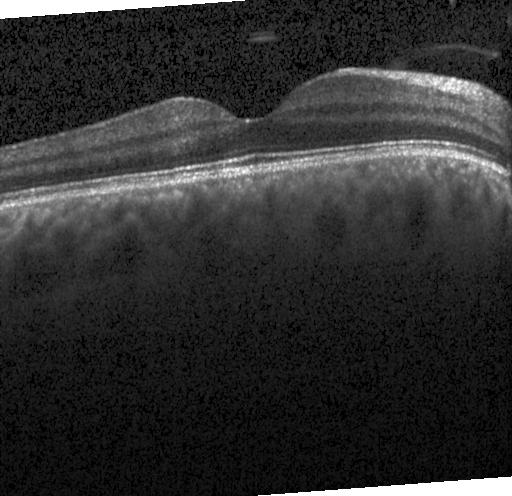
Spectral-domain OCT, retinal OCT B-scan — Impression: neither choroidal neovascularization, diabetic macular edema, nor drusen.